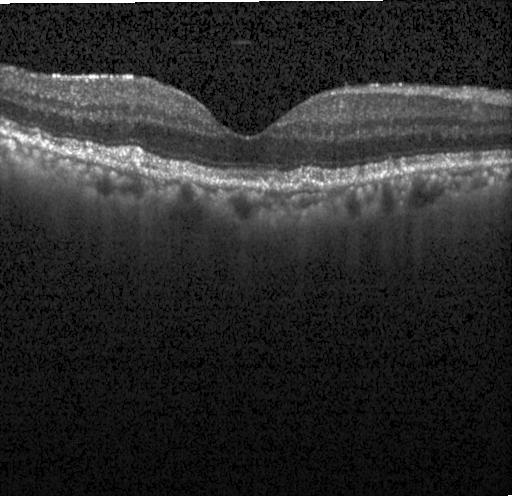 Optical coherence tomography B-scan. Horizontal scan through the fovea. Spectral-domain OCT. Heidelberg Spectralis
Macular OCT: drusen.